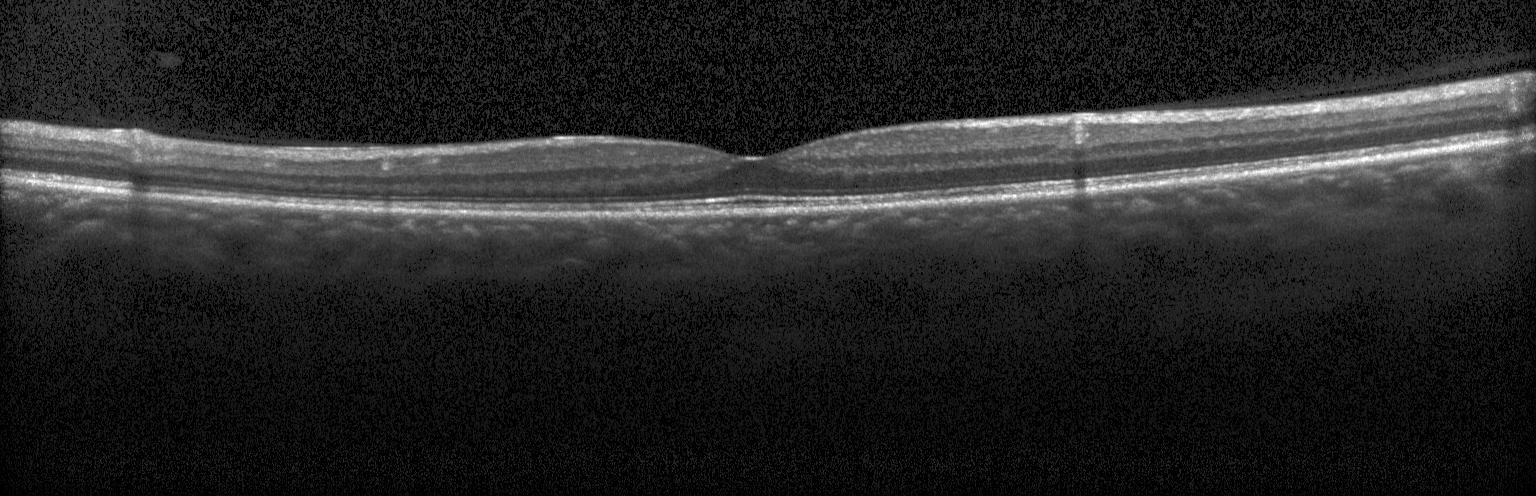

Finding: no CNV, no DME, and no drusen.